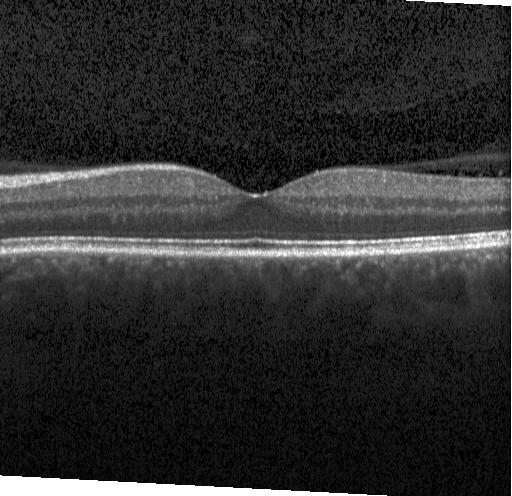
Optical coherence tomography scan
Macular OCT: no CNV, DME, or drusen.